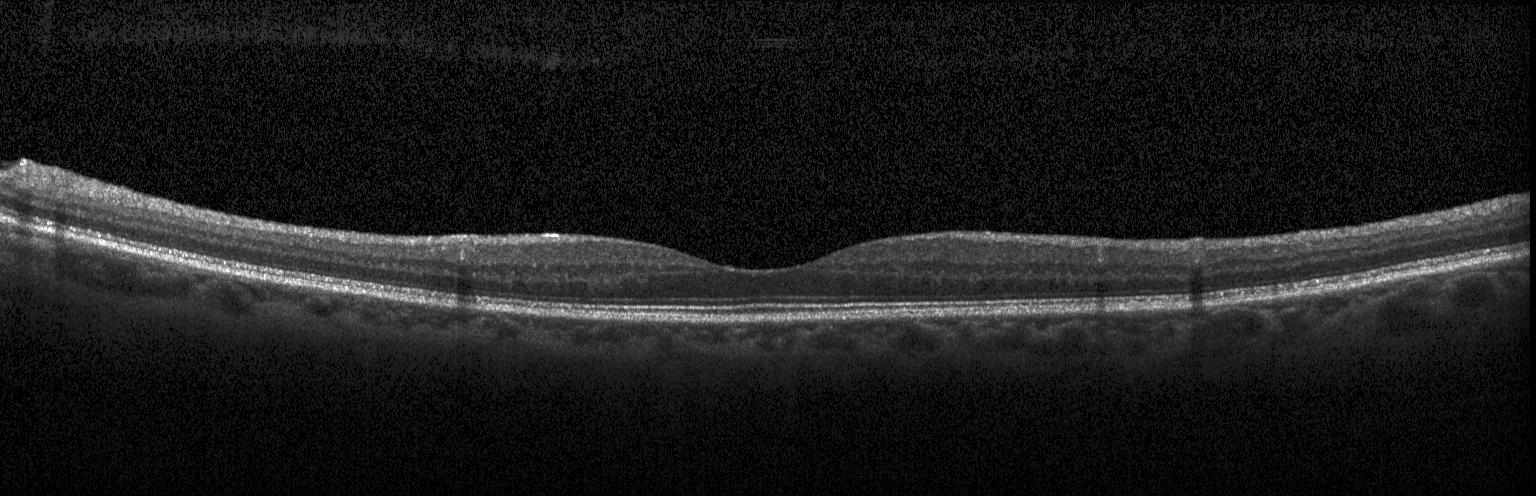 Heidelberg Spectralis · spectral-domain optical coherence tomography · optical coherence tomography scan
Impression: no evidence of choroidal neovascularization, diabetic macular edema, or drusen.